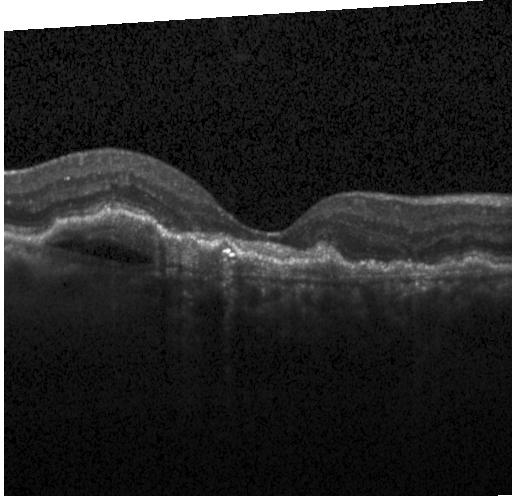 Spectral-domain OCT. Fovea-centered. OCT B-scan.
Finding: a choroidal neovascular membrane.